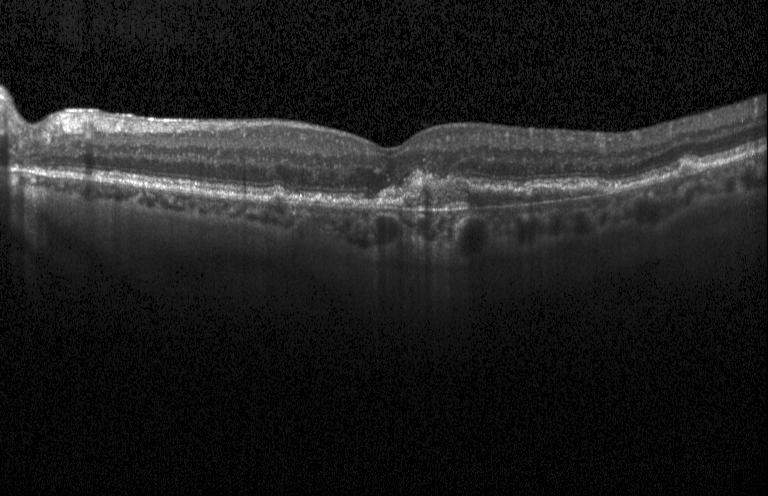

Finding: a choroidal neovascular membrane.